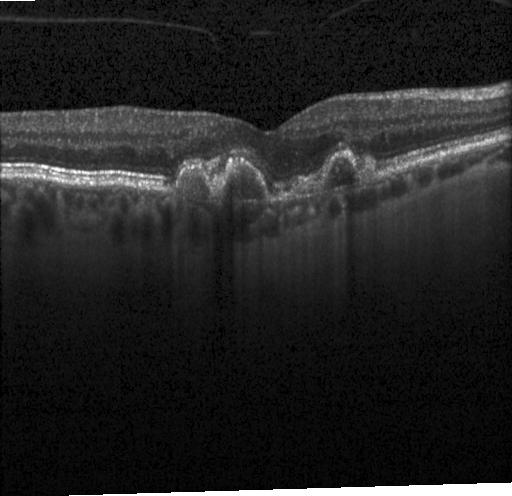 Spectral-domain OCT B-scan: choroidal neovascularization (CNV).